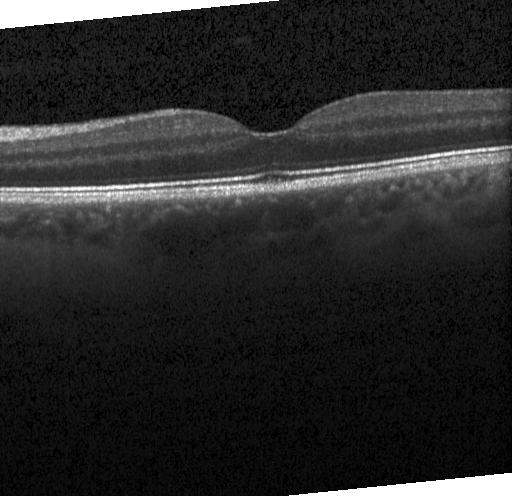
Optical coherence tomography B-scan · spectral-domain OCT · centered on the fovea · Heidelberg Spectralis OCT system — This B-scan demonstrates no choroidal neovascularization, no diabetic macular edema, and no drusen.